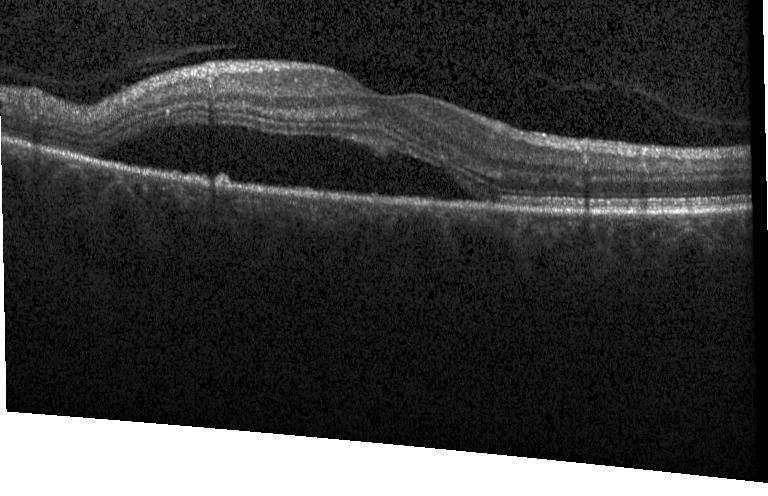 Impression: choroidal neovascularization (CNV).